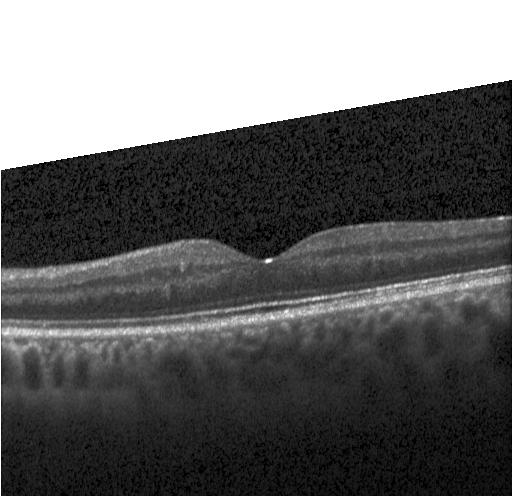

The scan shows no choroidal neovascularization, diabetic macular edema, or drusen.